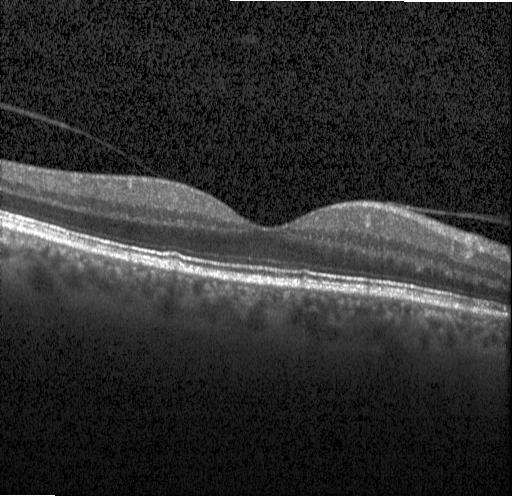

Acquired on a Heidelberg Spectralis. Horizontal scan through the fovea. Retinal OCT cross-section.
Multiple drusen.